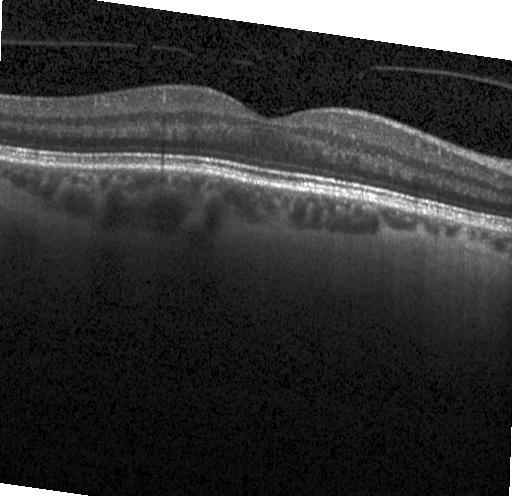 SD-OCT; retinal OCT B-scan; Heidelberg Spectralis OCT system — Diagnosis: no choroidal neovascularization, diabetic macular edema, or drusen.